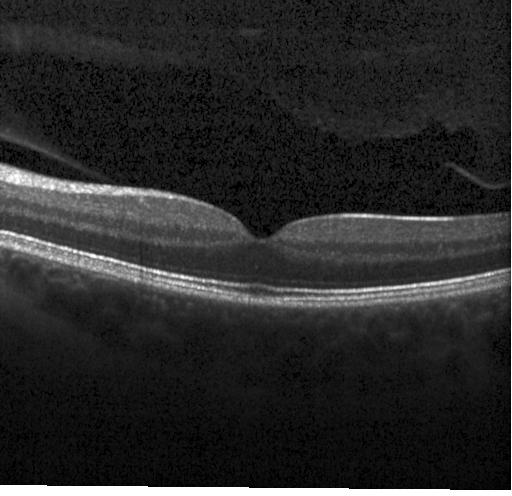
Optical coherence tomography scan — OCT finding: neither CNV, DME, nor drusen.